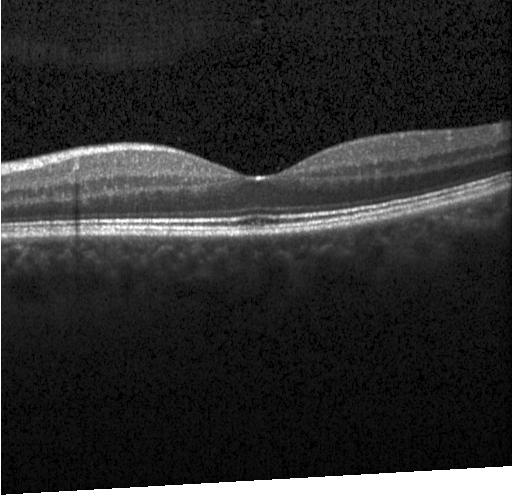 Spectral-domain optical coherence tomography; retinal OCT B-scan; acquired on a Heidelberg Spectralis; horizontal scan through the fovea
This B-scan demonstrates neither choroidal neovascularization, diabetic macular edema, nor drusen.